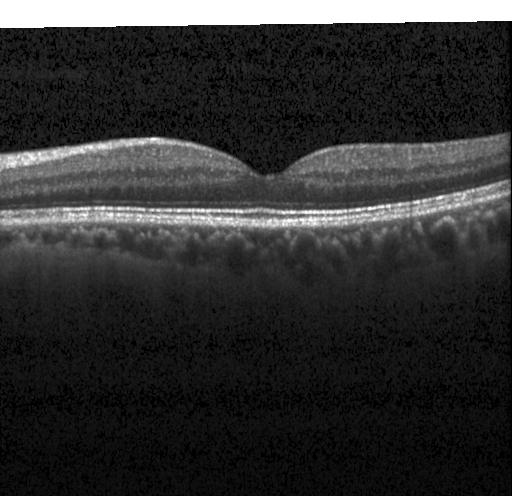 Finding: no CNV, DME, or drusen.